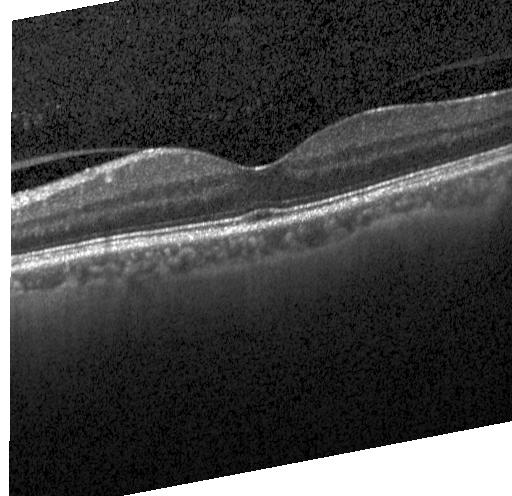

Spectral-domain optical coherence tomography, Heidelberg Spectralis OCT system, centered on the fovea, OCT B-scan. OCT finding: no choroidal neovascularization, diabetic macular edema, or drusen.